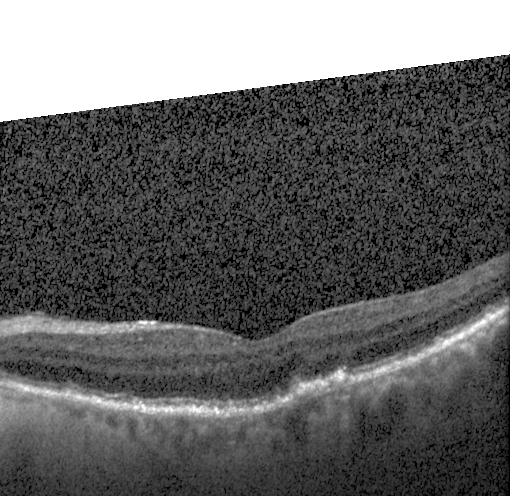

Instrument: Heidelberg Spectralis. Centered on the fovea. OCT line scan. SD-OCT. OCT finding: choroidal neovascularization.